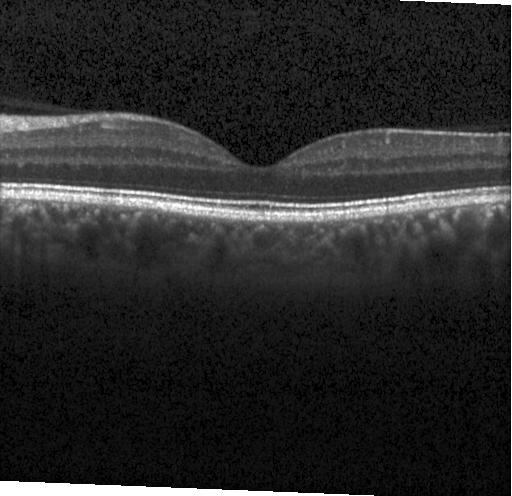
Instrument: Heidelberg Spectralis; horizontal scan through the fovea; OCT B-scan.
Impression: neither choroidal neovascularization, diabetic macular edema, nor drusen.